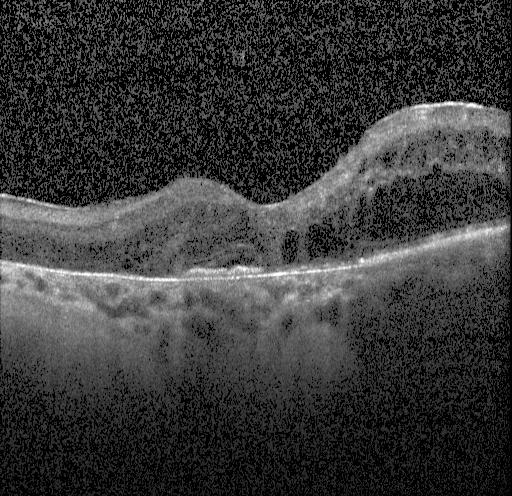

The scan shows a choroidal neovascular membrane.